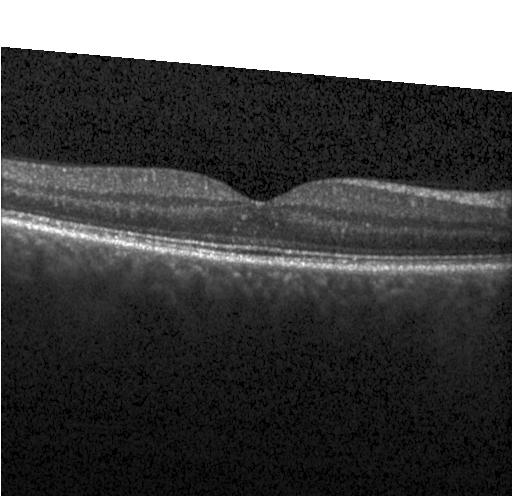 Spectral-domain optical coherence tomography · optical coherence tomography scan · through the macula. The scan shows no evidence of choroidal neovascularization, diabetic macular edema, or drusen.